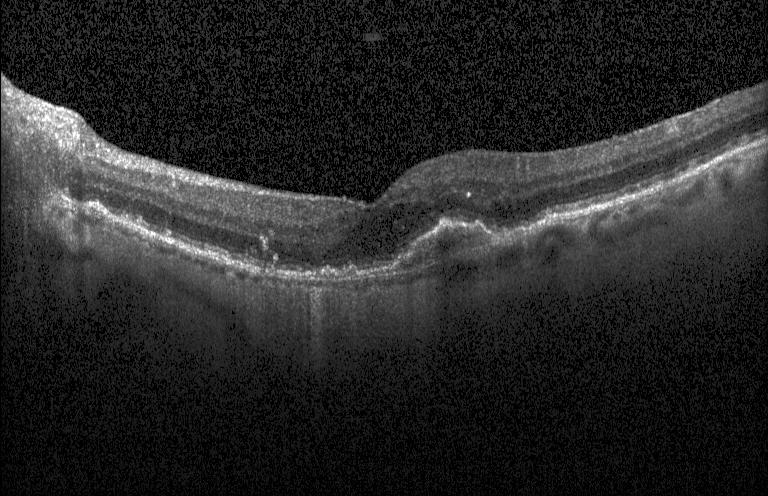 Finding: a choroidal neovascular membrane.